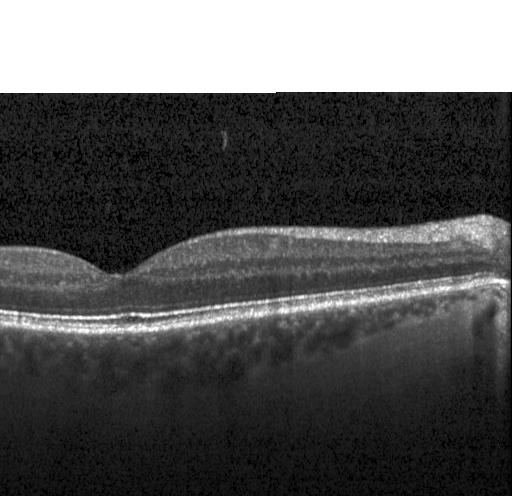

Optical coherence tomography scan · Heidelberg Spectralis · spectral-domain OCT — No choroidal neovascularization, no diabetic macular edema, and no drusen.